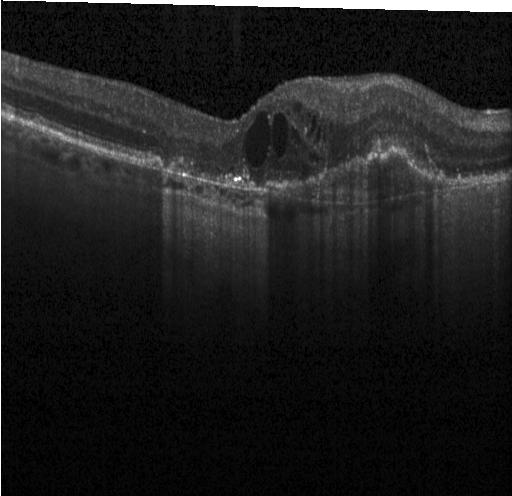
Finding: choroidal neovascularization.